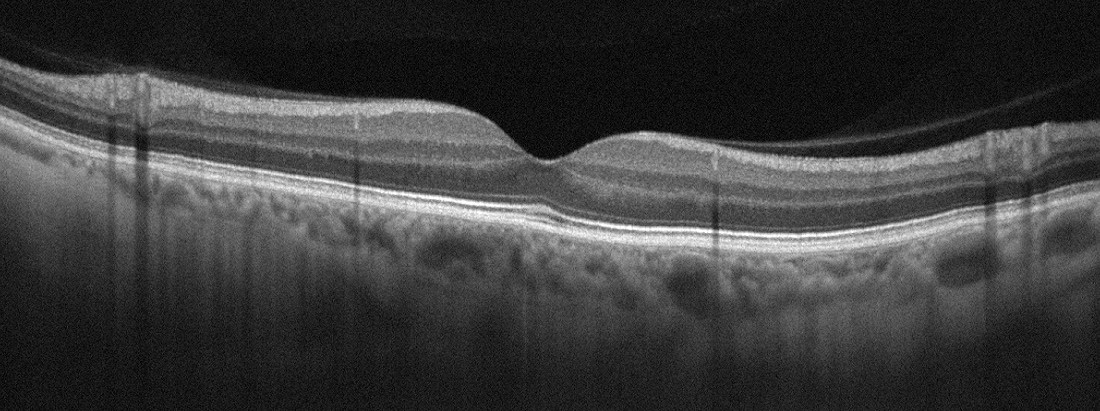

OCT line scan · instrument: Optovue Avanti RTVue XR — The scan shows no evidence of AMD, DME, ERM, RAO, RVO, or VID.